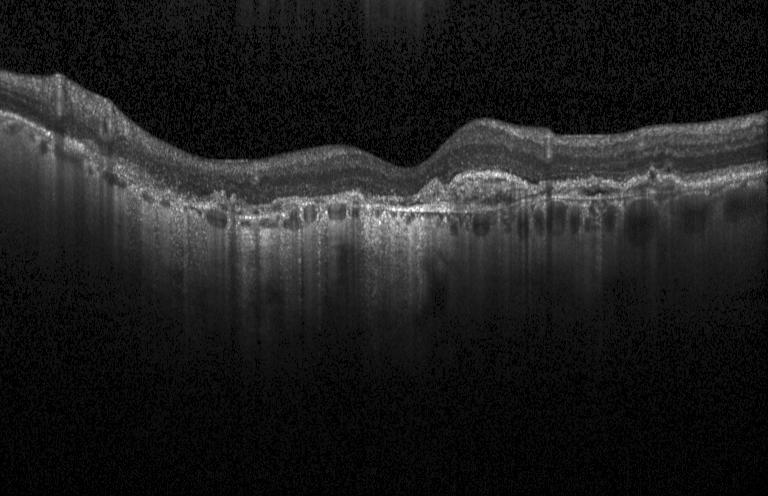 Finding: choroidal neovascularization.